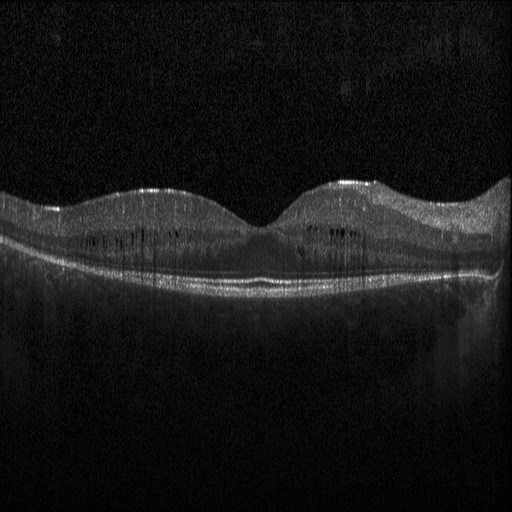

The scan shows diabetic macular edema (DME).